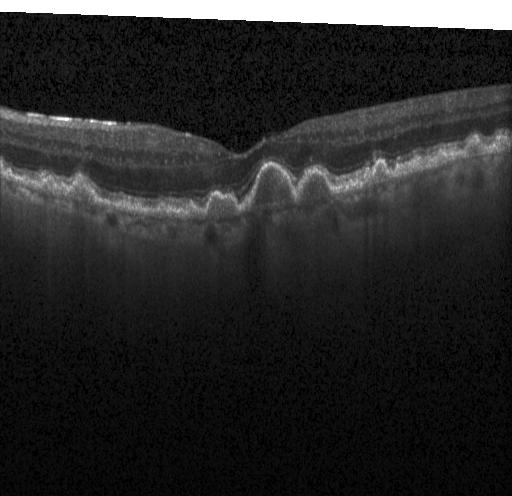 Instrument: Heidelberg Spectralis, OCT line scan, fovea-centered, spectral-domain OCT. Dx: multiple drusen.